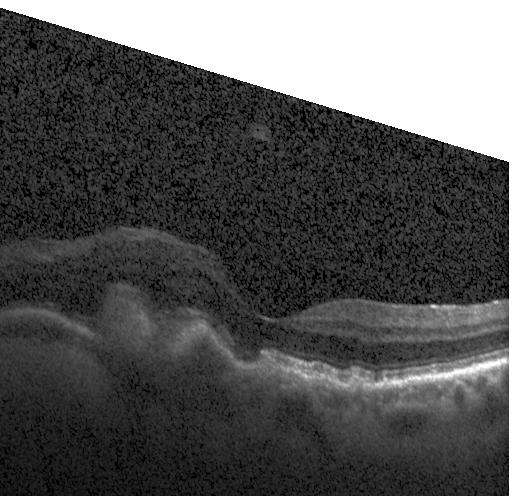
Retinal OCT B-scan
A choroidal neovascular membrane.